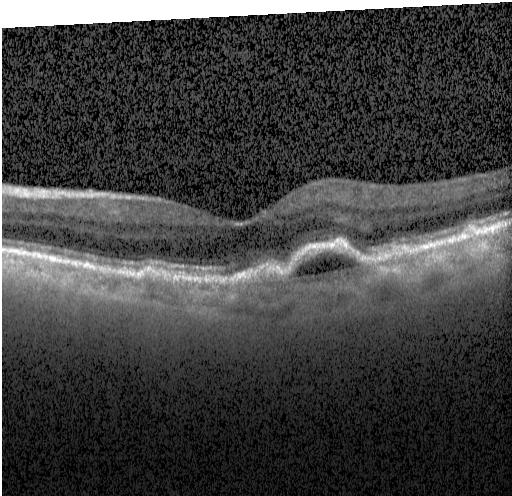 OCT line scan, acquired on a Heidelberg Spectralis, horizontal scan through the fovea, spectral-domain optical coherence tomography
OCT finding: choroidal neovascularization (CNV).